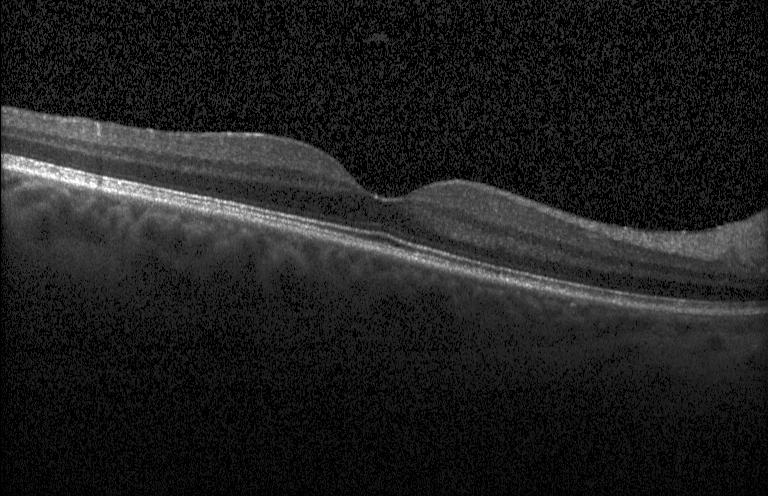

OCT B-scan.
Diagnosis: no CNV, DME, or drusen.